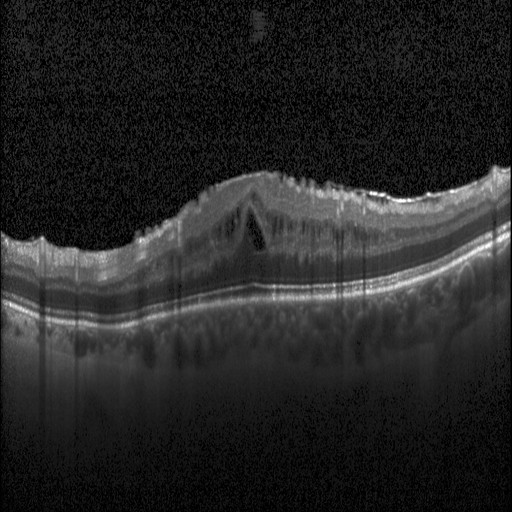

OCT scan showing diabetic macular edema.